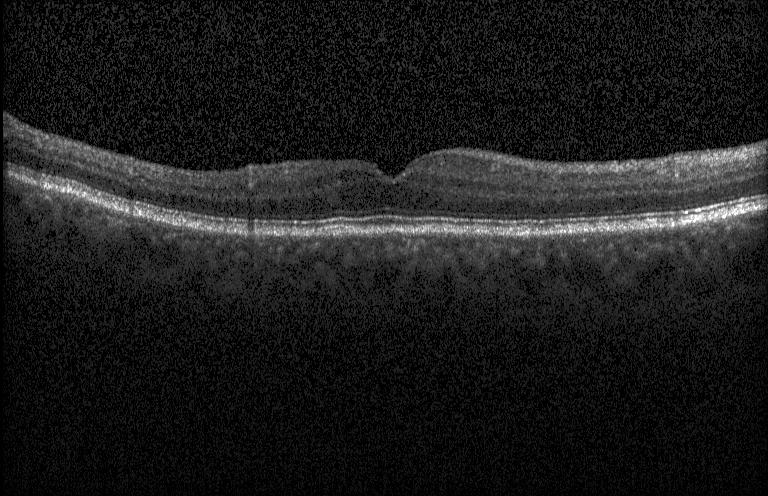
Retinal OCT B-scan, Heidelberg Spectralis OCT system, through the macula
Neither CNV, DME, nor drusen.